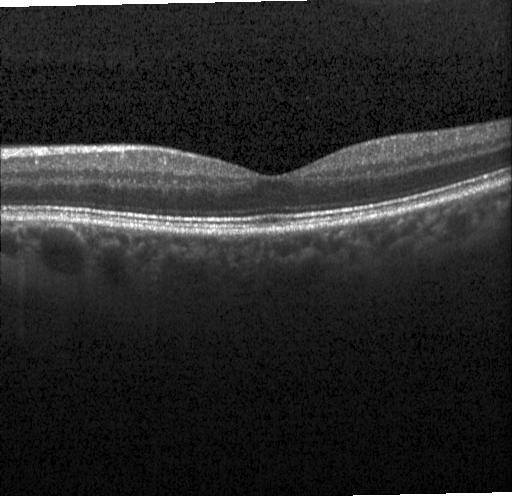
Dx: no choroidal neovascularization, diabetic macular edema, or drusen.